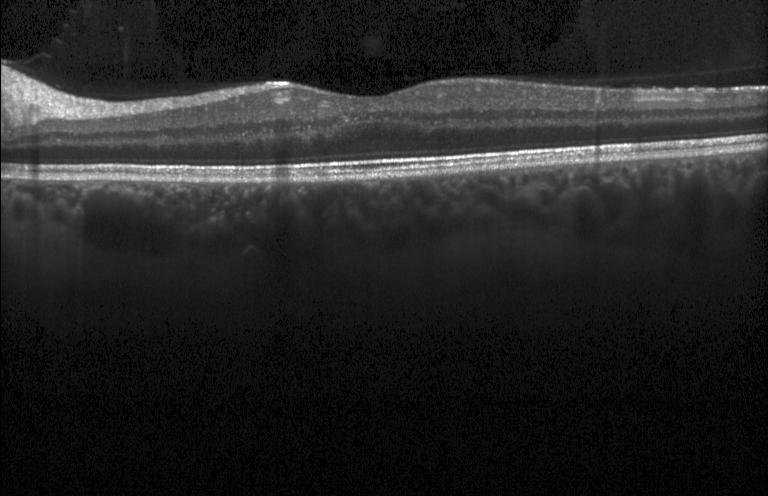 Macular OCT: no evidence of CNV, DME, or drusen.